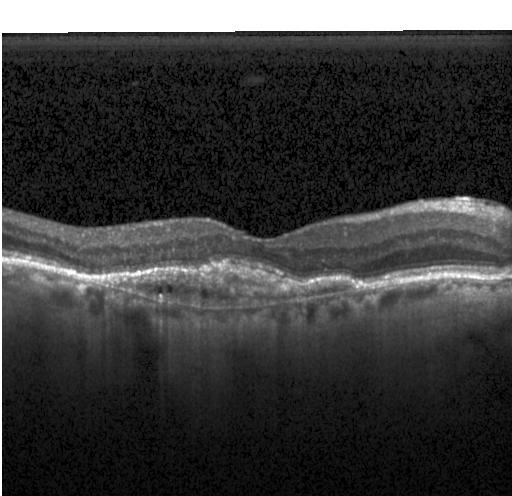 Macular OCT: choroidal neovascularization.